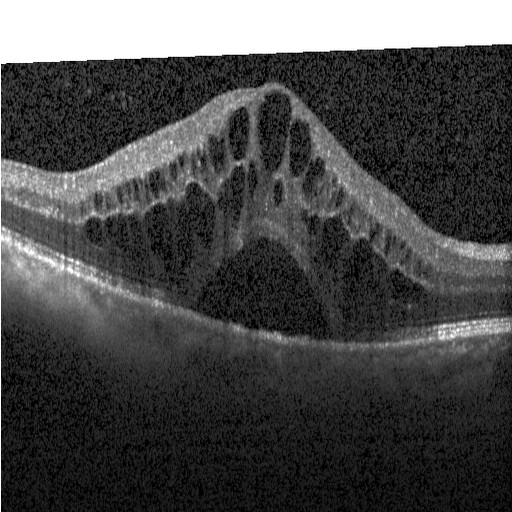 Optical coherence tomography B-scan
The scan shows diabetic macular edema.